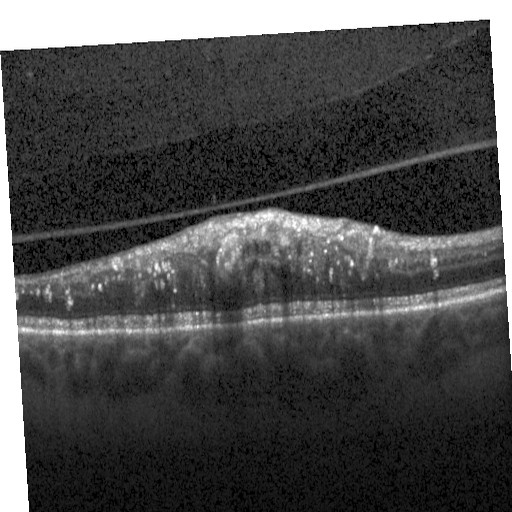
Finding: diabetic macular edema.